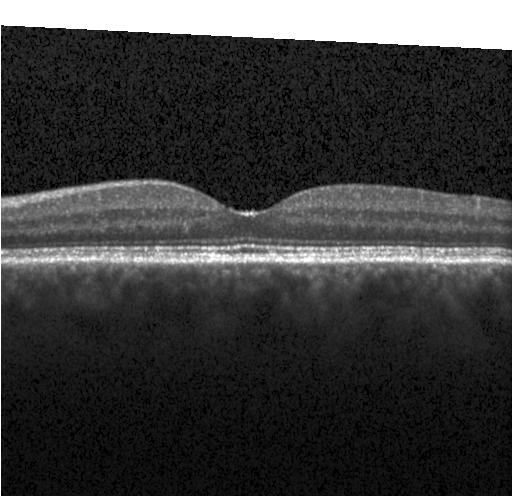 Through the macula; spectral-domain OCT; retinal OCT cross-section — Diagnosis: neither CNV, DME, nor drusen.